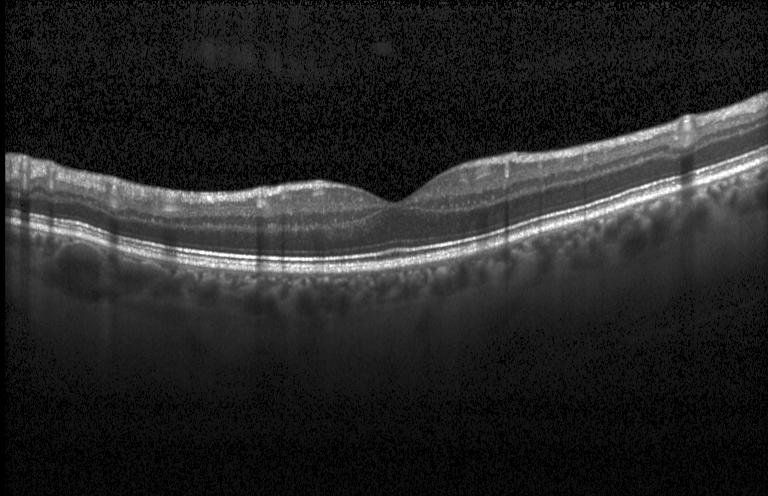
Optical coherence tomography B-scan. Instrument: Heidelberg Spectralis
Dx: neither choroidal neovascularization, diabetic macular edema, nor drusen.